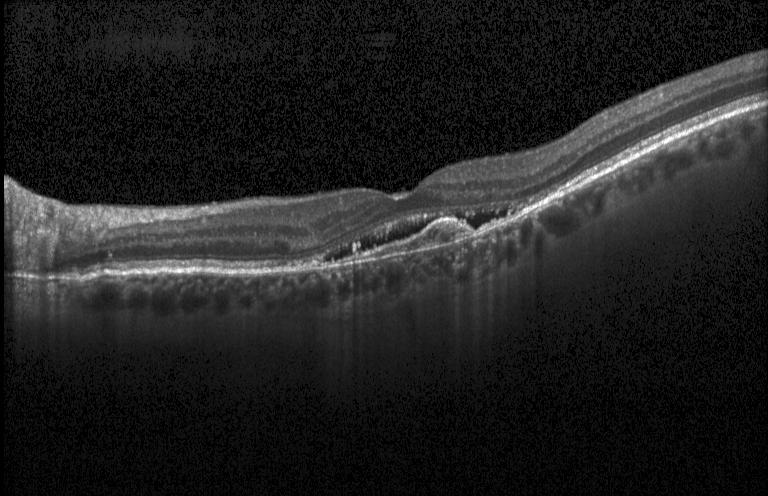
SD-OCT · retinal OCT B-scan — Diagnosis: a choroidal neovascular membrane.